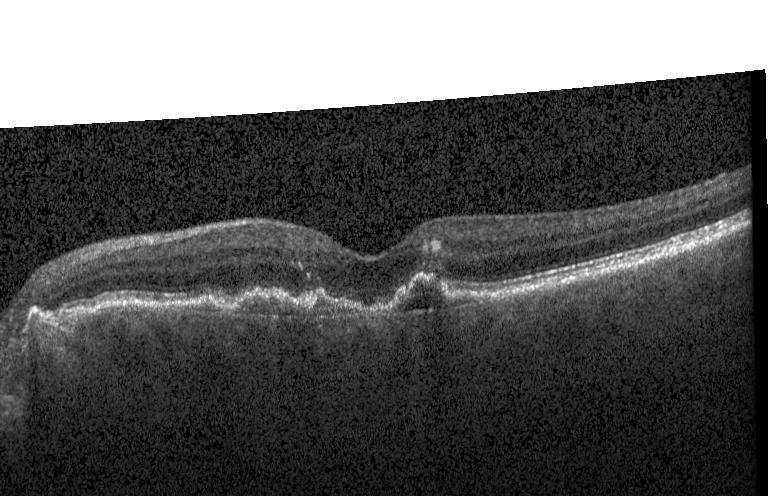

OCT scan showing CNV.